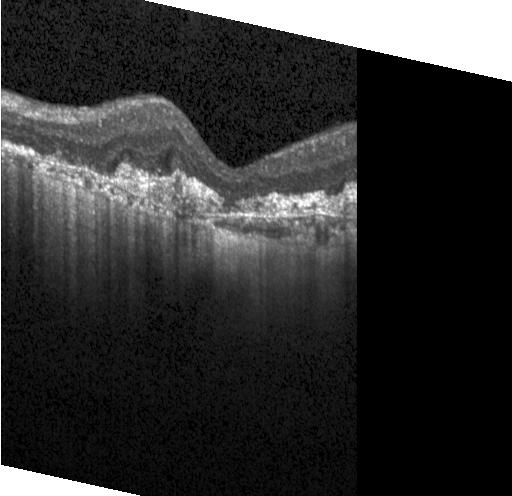

Optical coherence tomography B-scan. Diagnosis: a choroidal neovascular membrane.